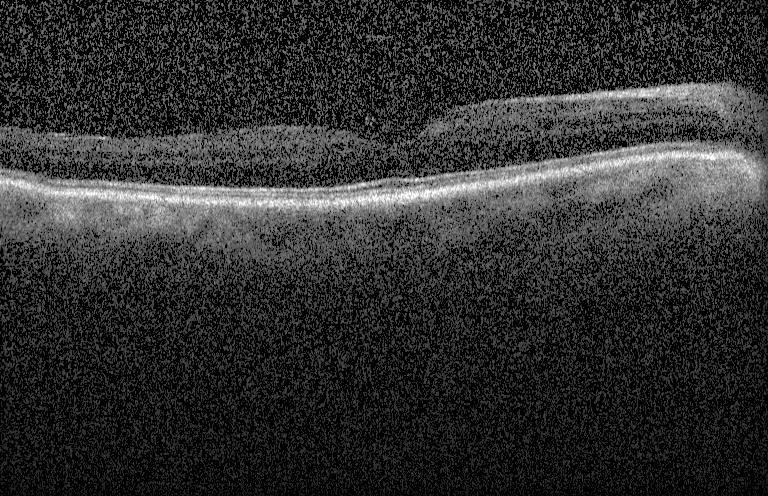 OCT scan showing no choroidal neovascularization, diabetic macular edema, or drusen.